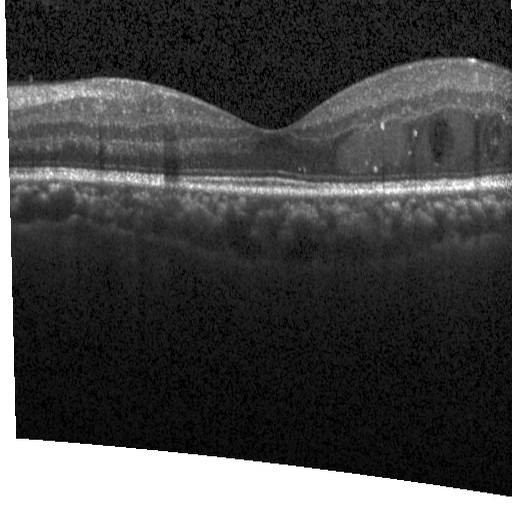 OCT B-scan; Heidelberg Spectralis; centered on the fovea; SD-OCT. The scan shows diabetic macular edema (DME).